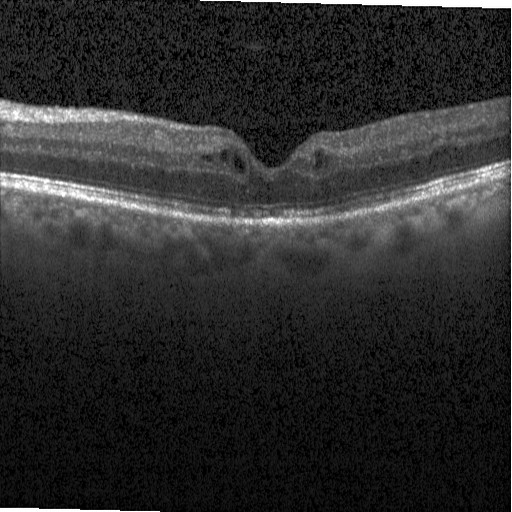 Heidelberg Spectralis, OCT line scan.
Finding: DME.